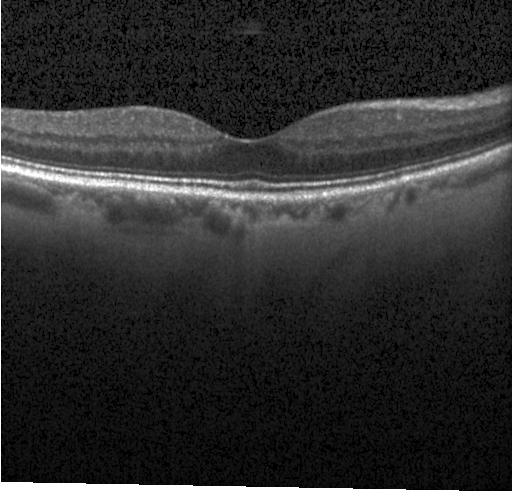

Impression: no choroidal neovascularization, diabetic macular edema, or drusen.